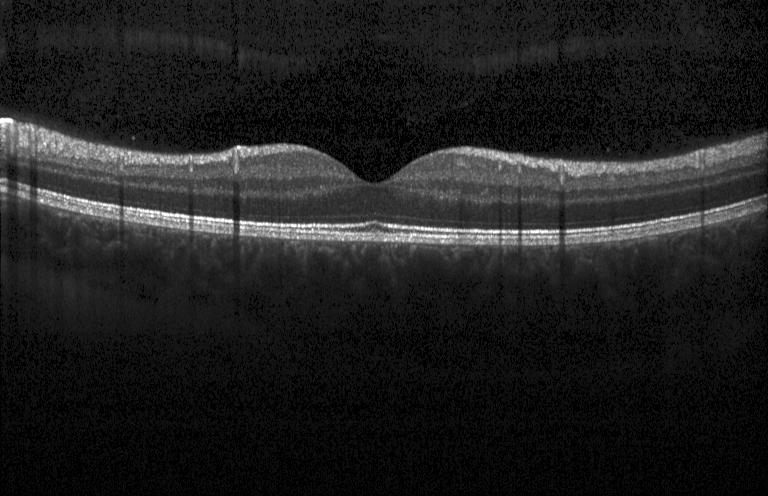 Impression: neither choroidal neovascularization, diabetic macular edema, nor drusen.